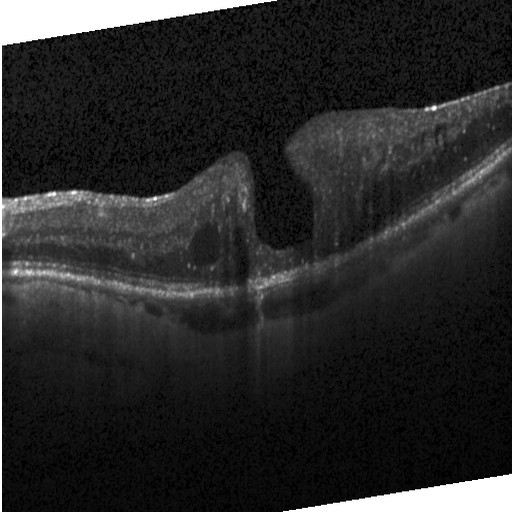
Impression: diabetic macular edema (DME).